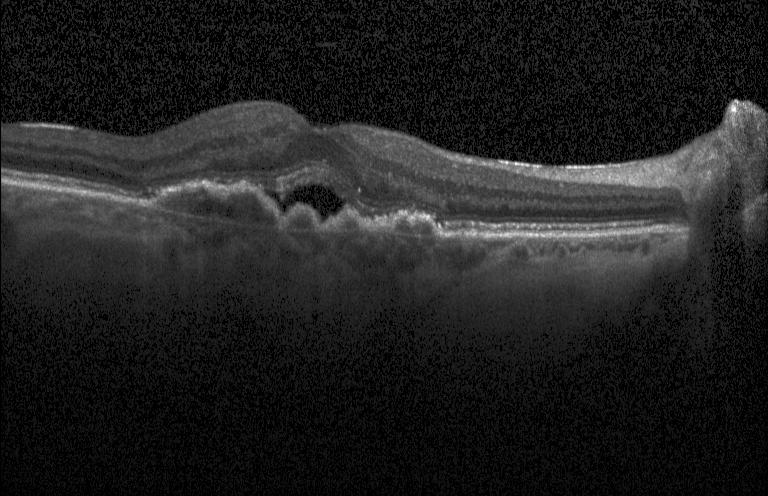

Heidelberg Spectralis OCT system · SD-OCT · macular scan · OCT line scan
Diagnosis: CNV.